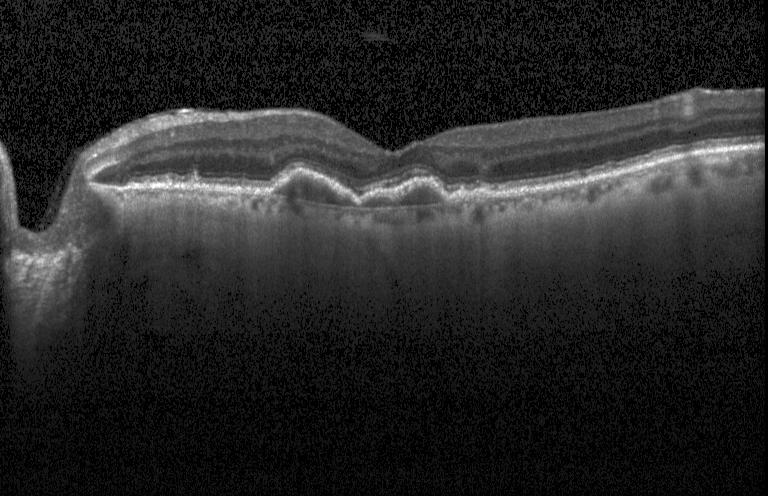 Optical coherence tomography scan. Horizontal scan through the fovea. Heidelberg Spectralis. Spectral-domain OCT — OCT finding: a choroidal neovascular membrane.